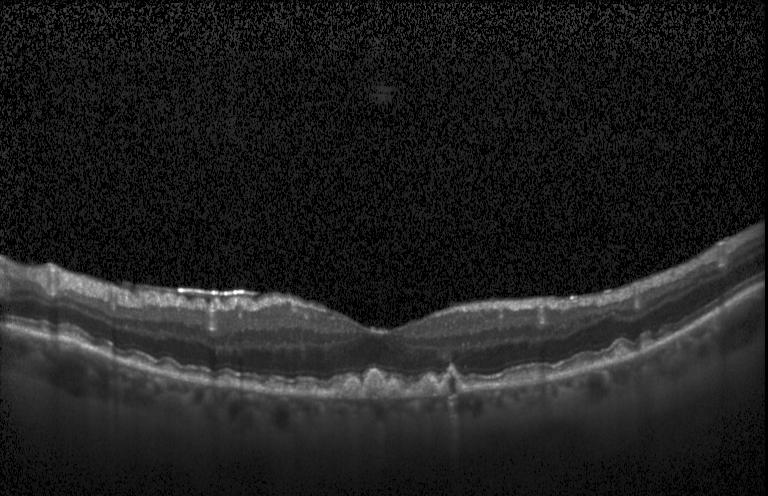
Diagnosis: multiple drusen.